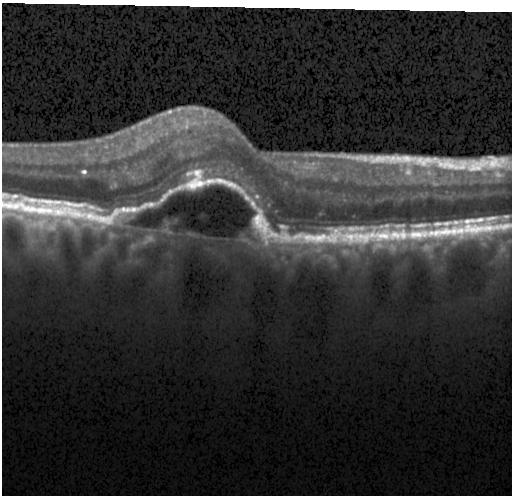 Assessment: CNV.